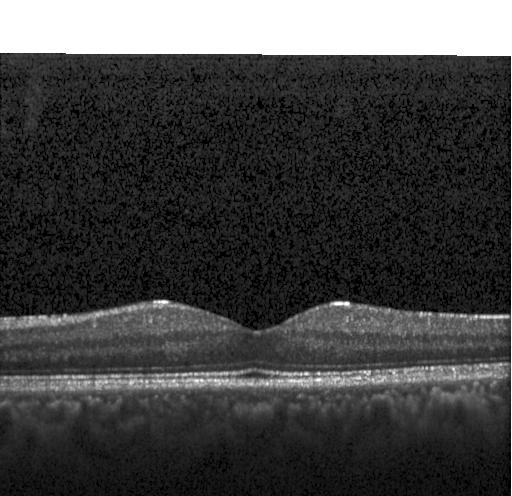
Retinal OCT cross-section — Finding: no evidence of CNV, DME, or drusen.